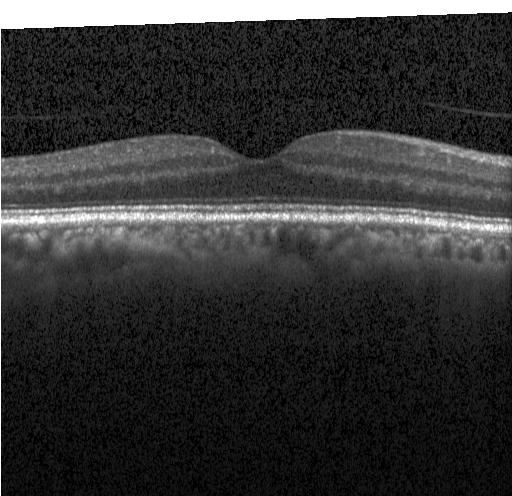
Spectral-domain optical coherence tomography. Optical coherence tomography scan. Acquired on a Heidelberg Spectralis.
Assessment: neither choroidal neovascularization, diabetic macular edema, nor drusen.